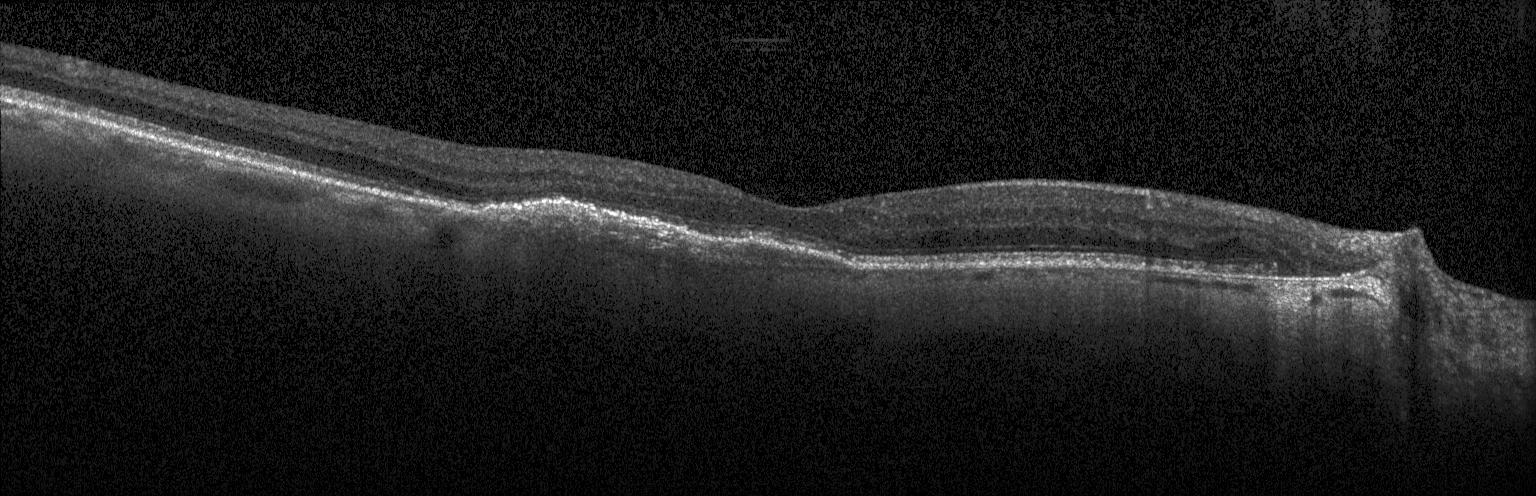

This B-scan demonstrates a choroidal neovascular membrane.